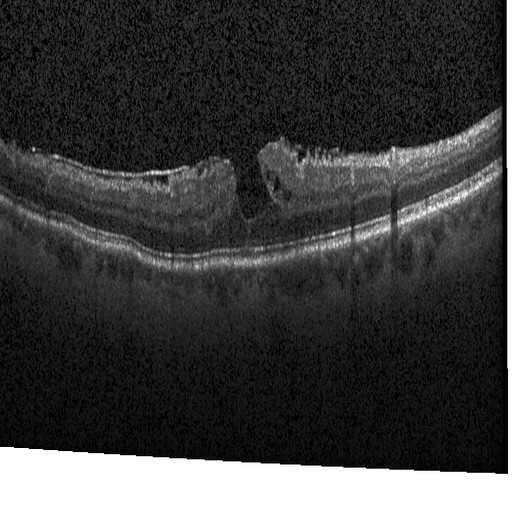 Optical coherence tomography scan. Finding: diabetic macular edema.